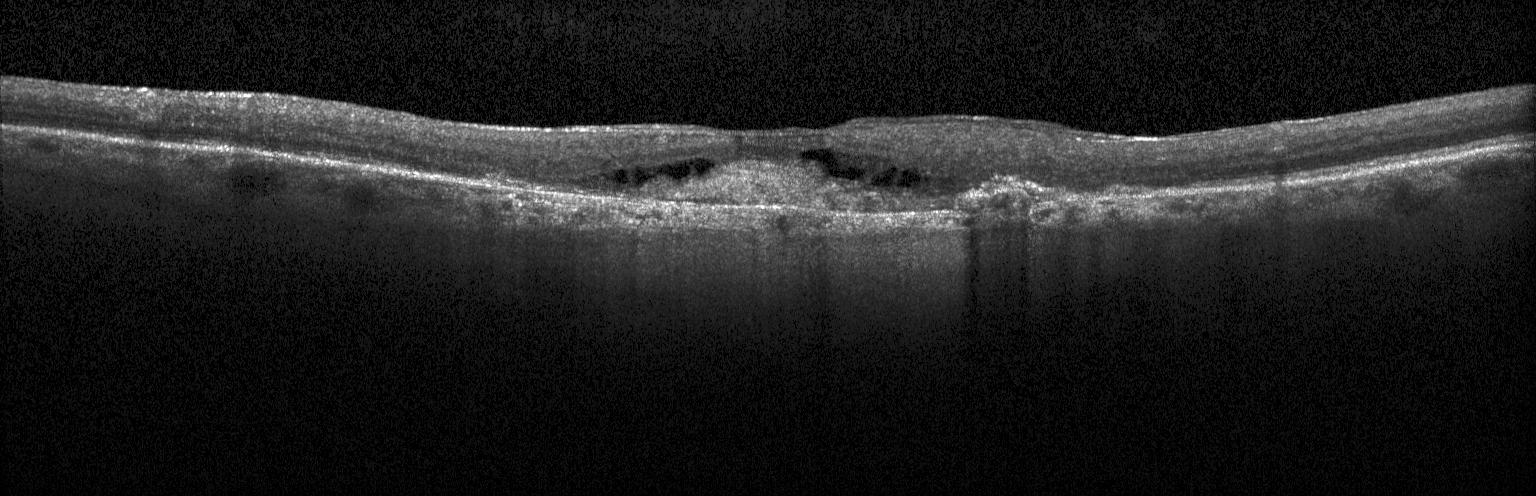 Optical coherence tomography B-scan; spectral-domain optical coherence tomography — Macular OCT: CNV.